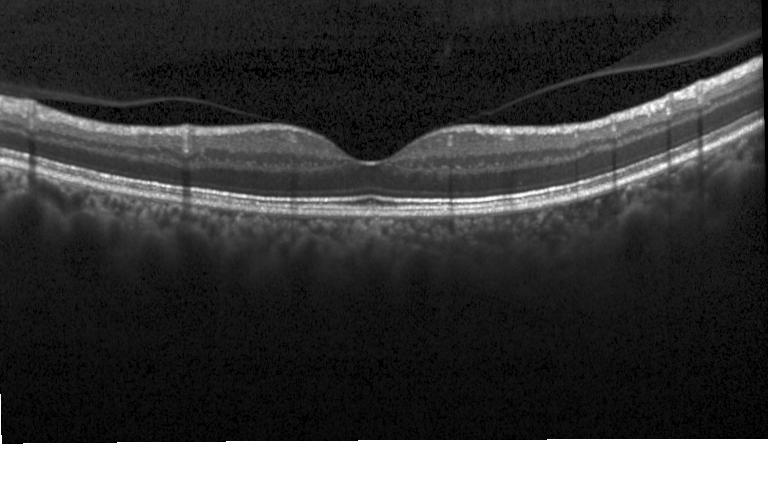
Impression: no CNV, no DME, and no drusen.